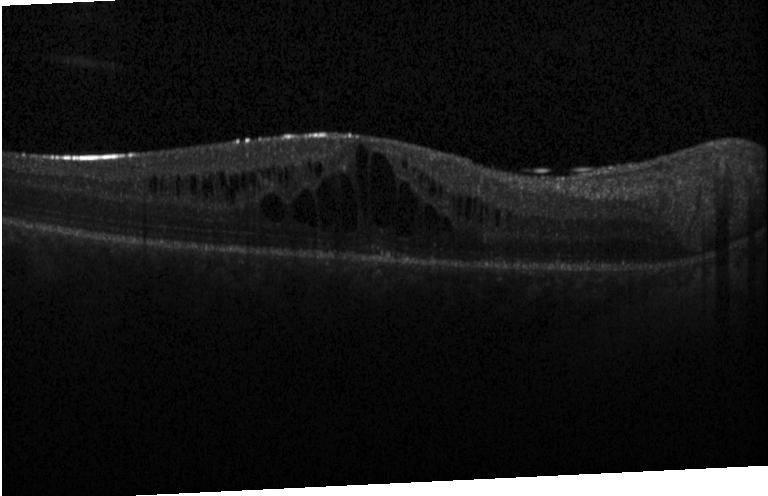 Diagnosis: diabetic macular edema.